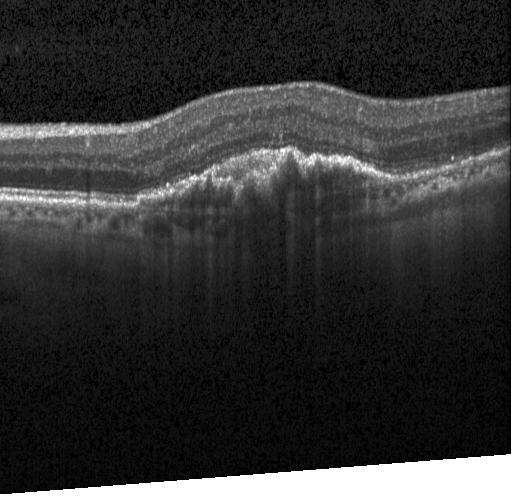
Instrument: Heidelberg Spectralis, macular scan, OCT B-scan. OCT finding: CNV.